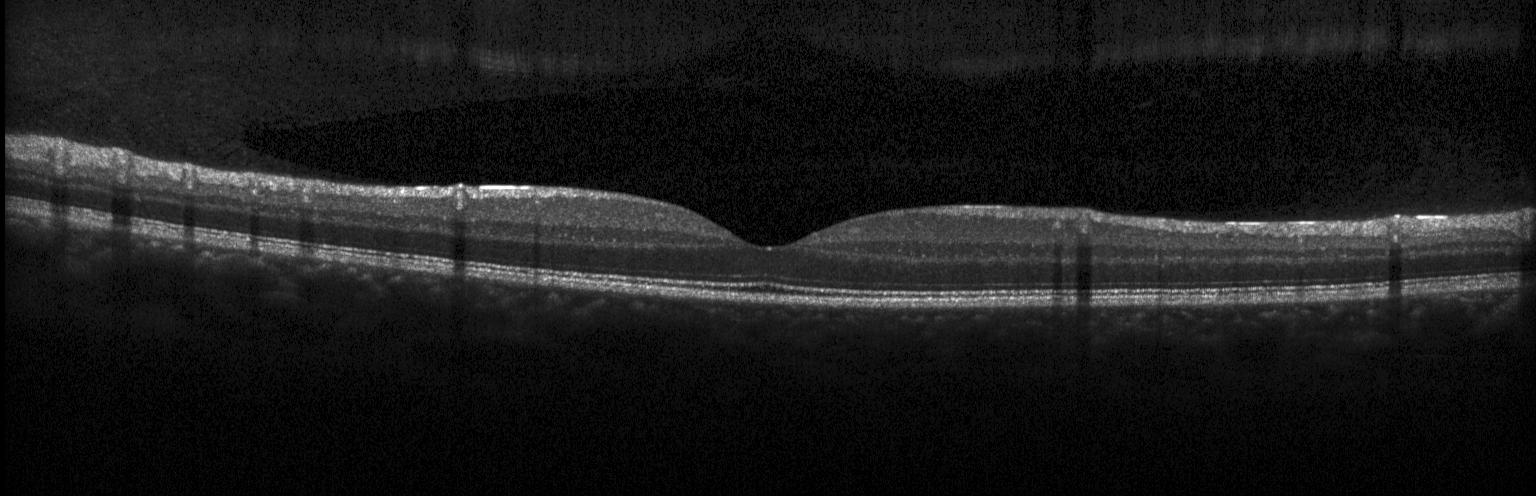 Optical coherence tomography scan. The scan shows no CNV, DME, or drusen.